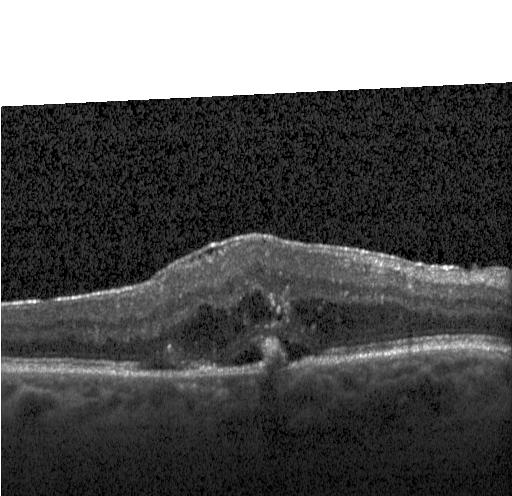
The scan shows a choroidal neovascular membrane.